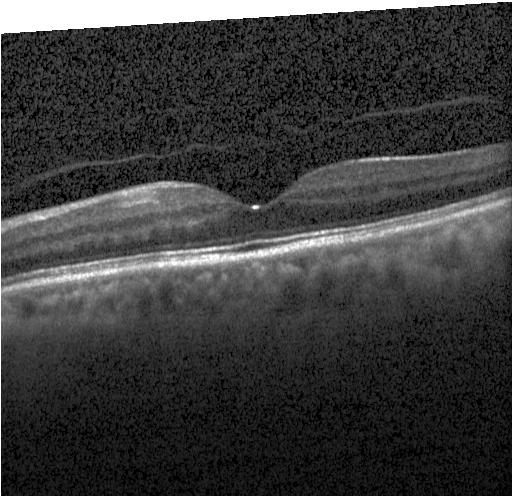
Retinal OCT cross-section, acquired on a Heidelberg Spectralis, spectral-domain OCT — Diagnosis: no choroidal neovascularization, diabetic macular edema, or drusen.